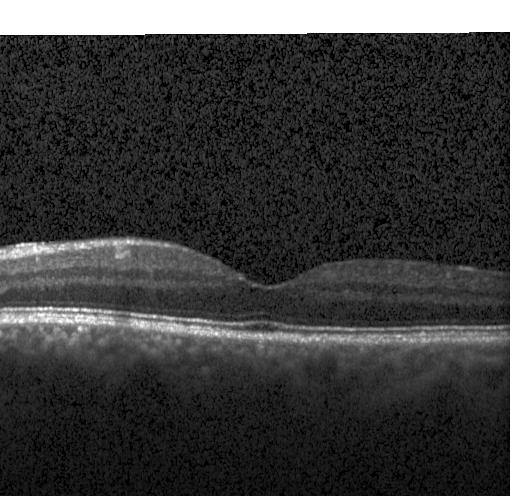 No evidence of choroidal neovascularization, diabetic macular edema, or drusen.